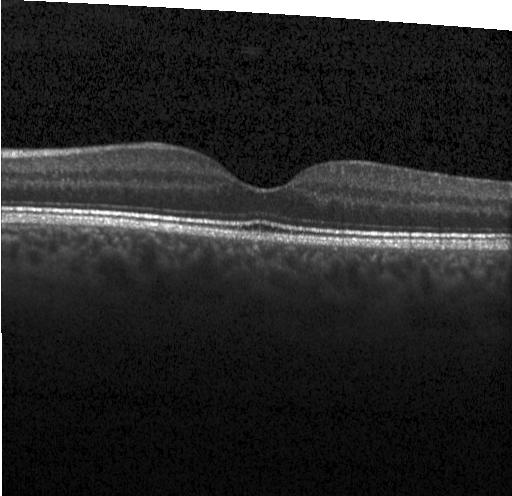
Optical coherence tomography scan.
Diagnosis: no choroidal neovascularization, diabetic macular edema, or drusen.